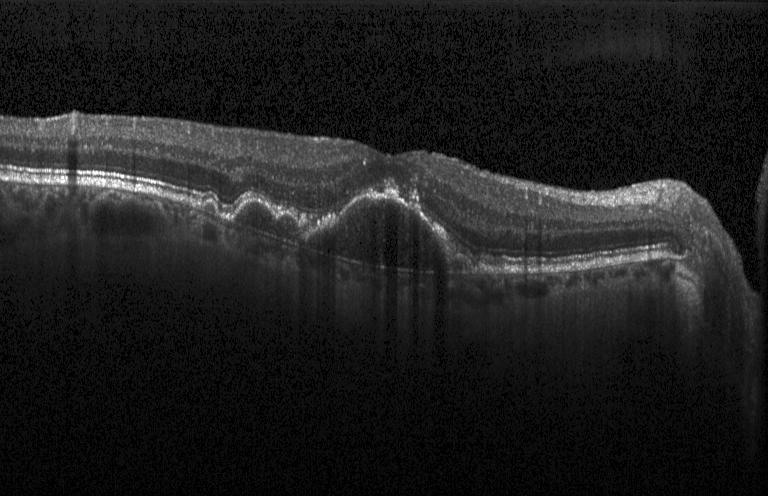
Diagnosis: choroidal neovascularization.